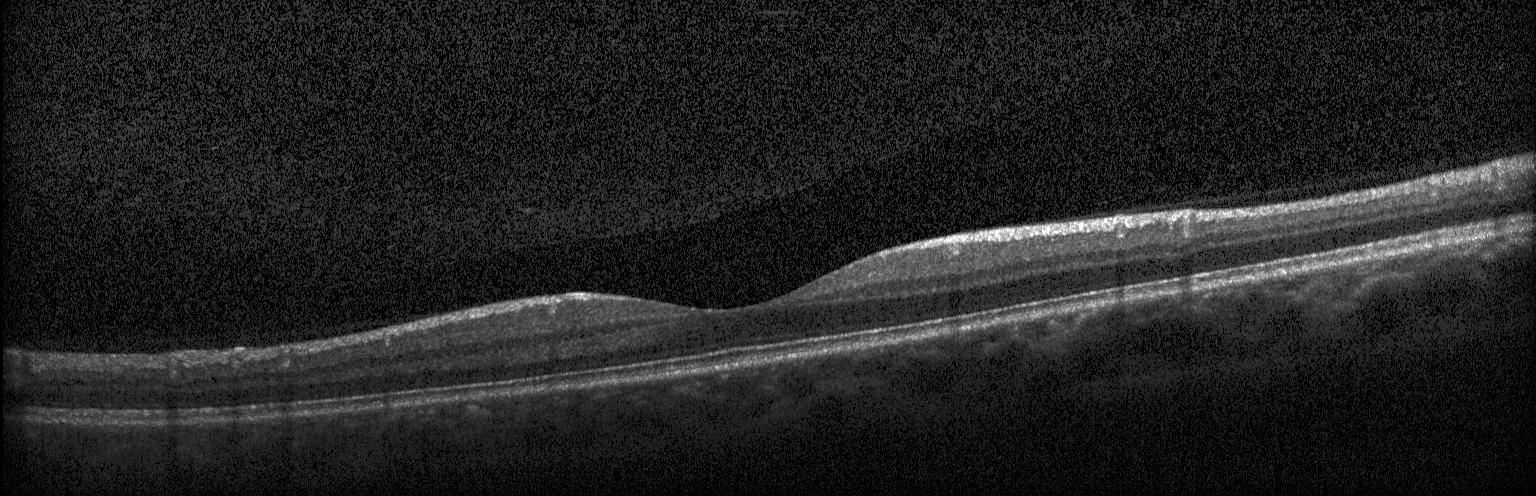

Optical coherence tomography B-scan, SD-OCT — No choroidal neovascularization, no diabetic macular edema, and no drusen.